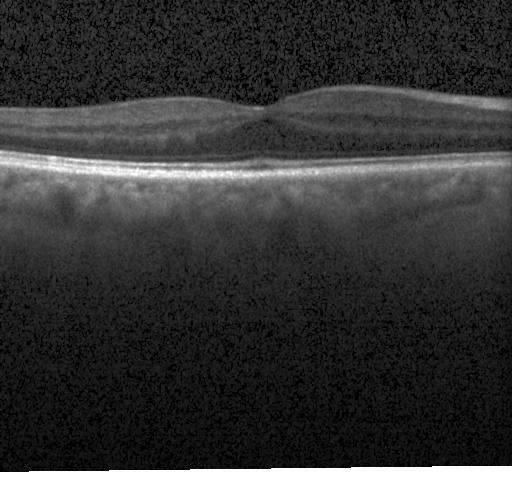 Retinal OCT B-scan.
OCT finding: neither CNV, DME, nor drusen.